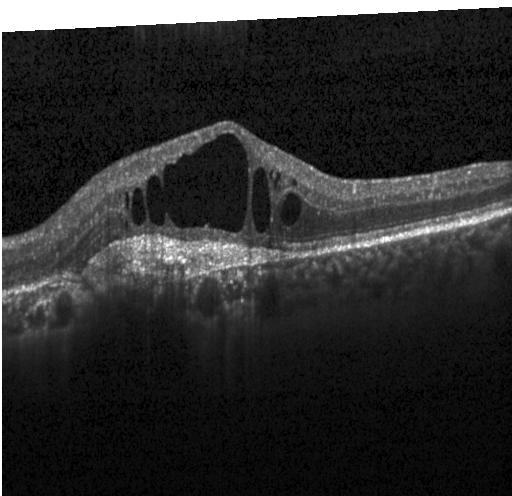 Macular scan · OCT B-scan. Macular OCT: a choroidal neovascular membrane.